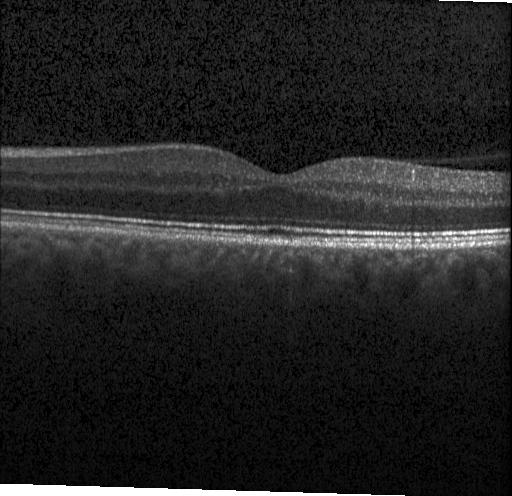 OCT finding: neither choroidal neovascularization, diabetic macular edema, nor drusen.